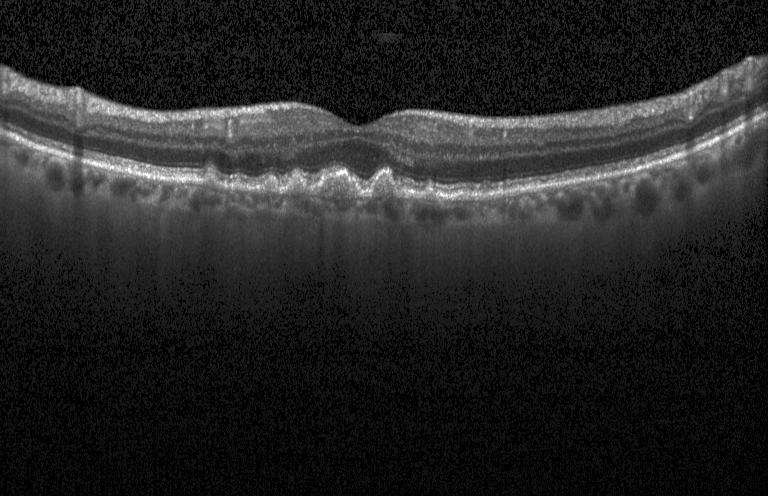

OCT finding: multiple drusen.